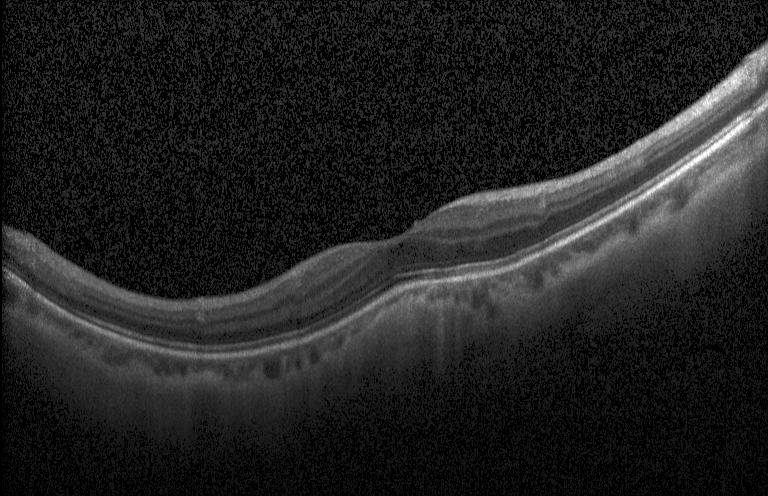 Instrument: Heidelberg Spectralis, spectral-domain OCT, optical coherence tomography B-scan — Dx: no choroidal neovascularization, diabetic macular edema, or drusen.